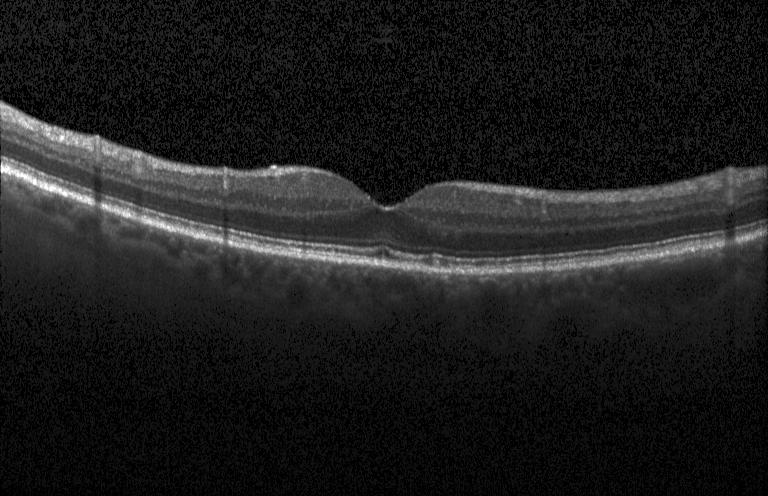 Optical coherence tomography scan — The scan shows no evidence of CNV, DME, or drusen.